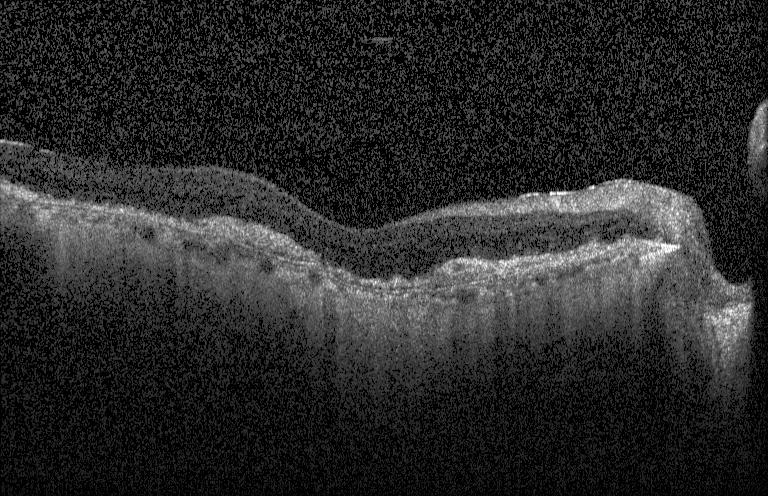

SD-OCT, optical coherence tomography B-scan.
Impression: a choroidal neovascular membrane.